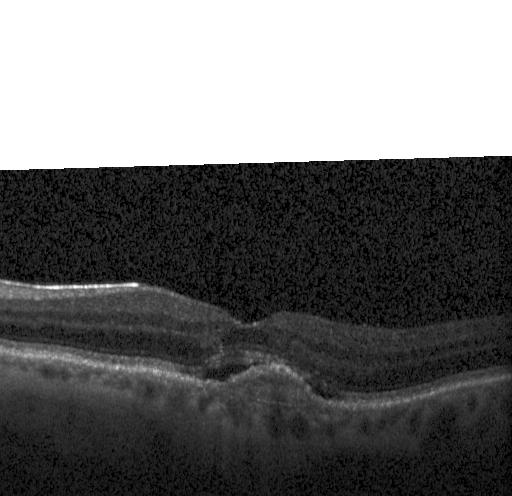

Retinal OCT cross-section showing CNV.